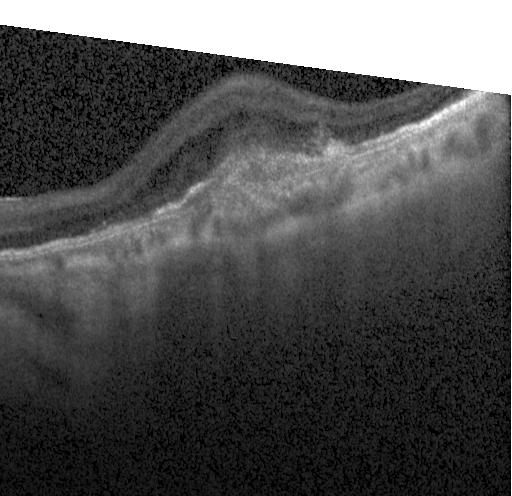

OCT line scan · SD-OCT · instrument: Heidelberg Spectralis.
Impression: a choroidal neovascular membrane.